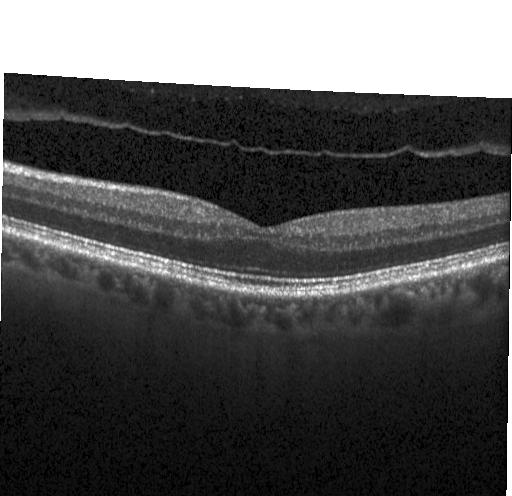
OCT line scan — Diagnosis: no evidence of choroidal neovascularization, diabetic macular edema, or drusen.